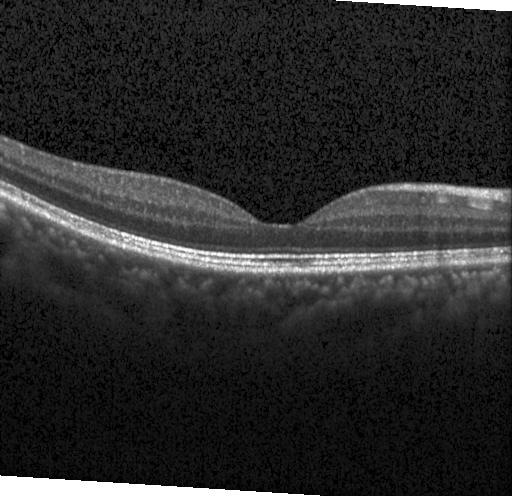 Macular OCT demonstrating no choroidal neovascularization, no diabetic macular edema, and no drusen.